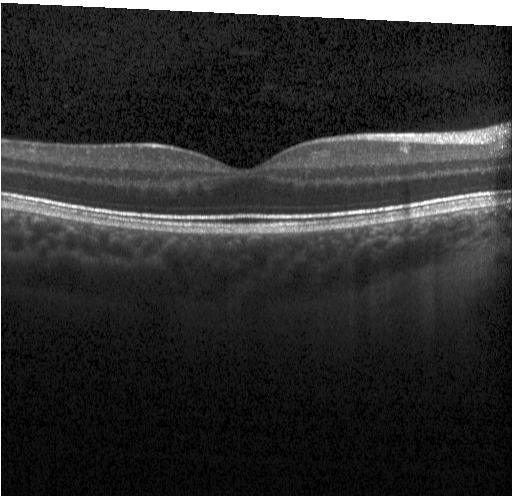

Macular scan. Spectral-domain OCT. Acquired on a Heidelberg Spectralis. Optical coherence tomography B-scan. Diagnosis: no evidence of choroidal neovascularization, diabetic macular edema, or drusen.